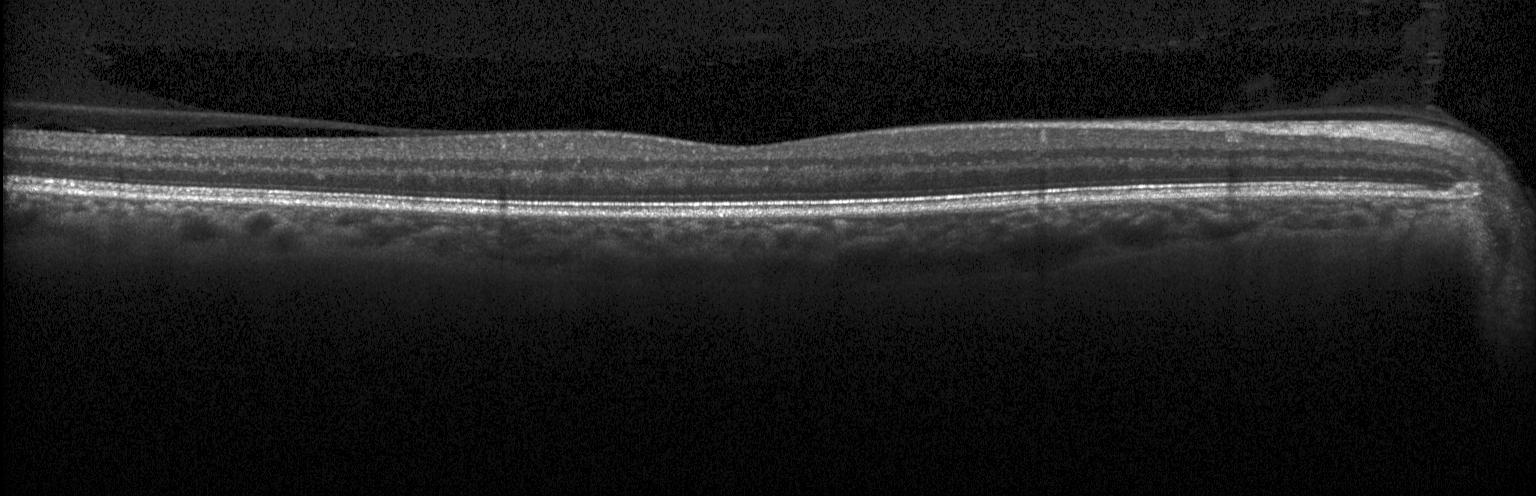 Optical coherence tomography scan — Macular OCT: no evidence of choroidal neovascularization, diabetic macular edema, or drusen.